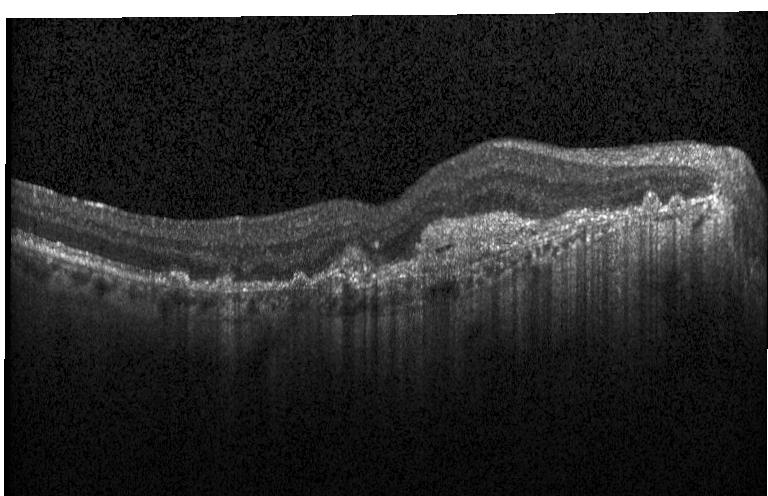 This B-scan demonstrates a choroidal neovascular membrane.